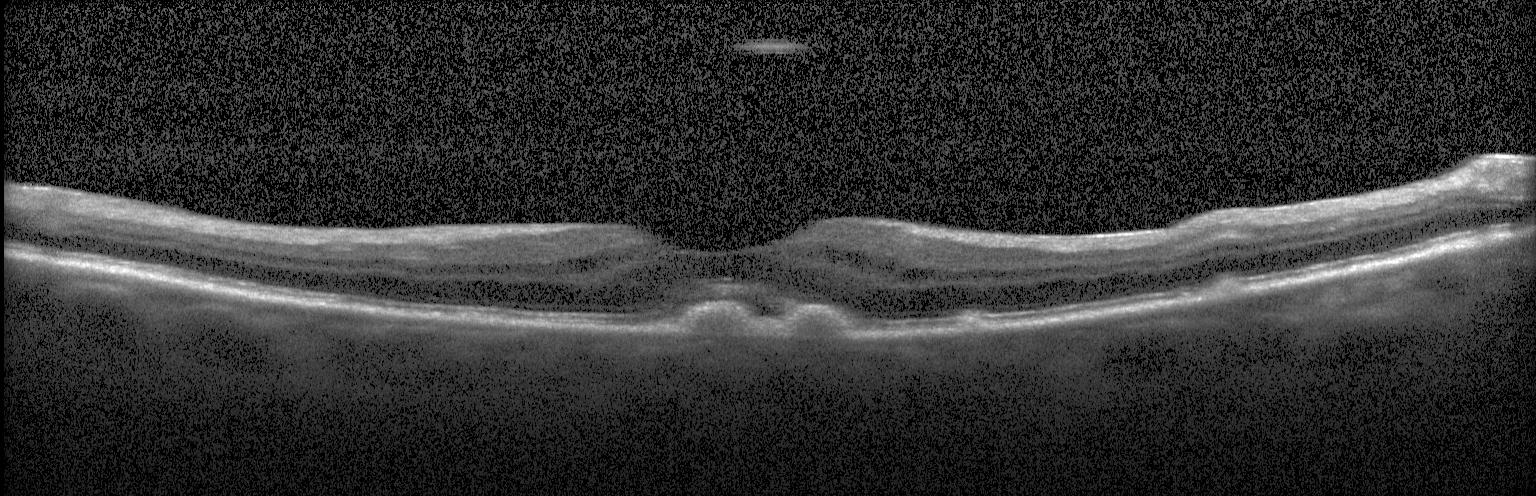

Spectral-domain optical coherence tomography. Instrument: Heidelberg Spectralis. Optical coherence tomography scan.
Finding: choroidal neovascularization (CNV).